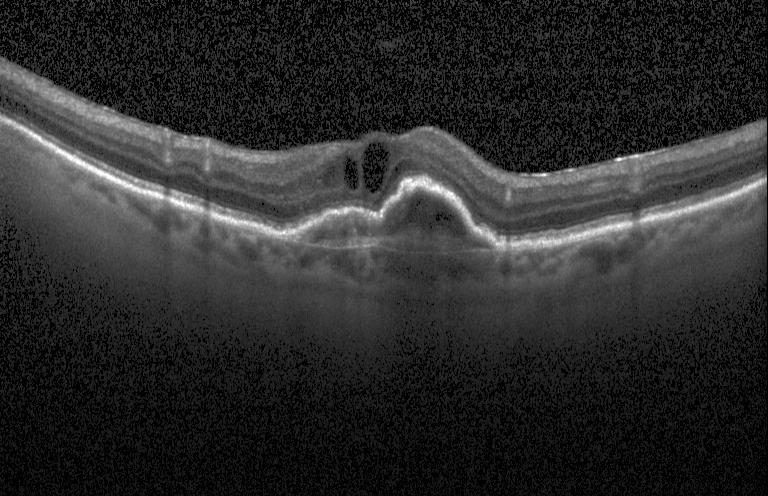

Retinal OCT cross-section
A choroidal neovascular membrane.